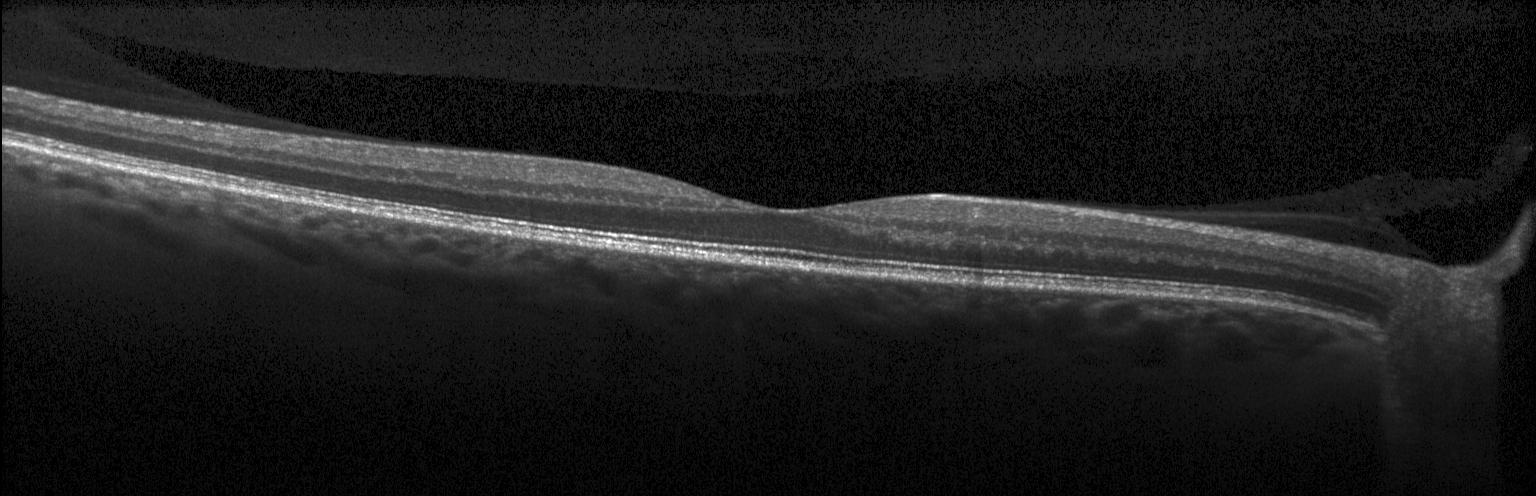 Through the macula; Heidelberg Spectralis OCT system; OCT line scan; spectral-domain OCT
Diagnosis: no evidence of CNV, DME, or drusen.